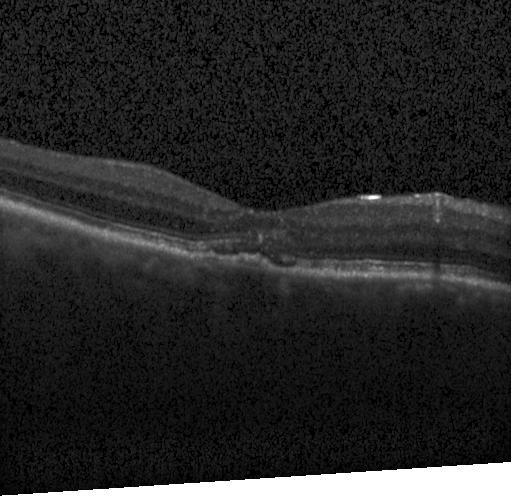

Finding: a choroidal neovascular membrane.